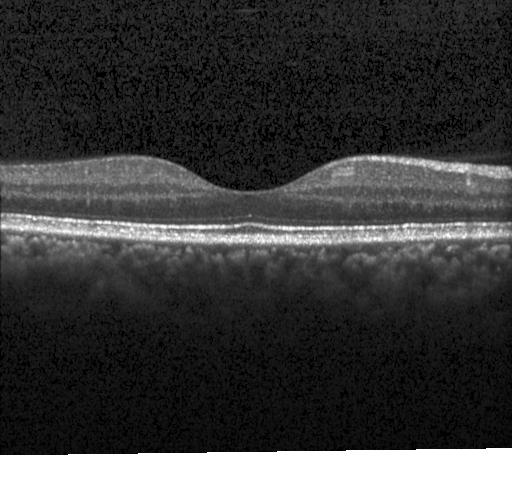 Heidelberg Spectralis OCT system. Optical coherence tomography scan — Assessment: neither choroidal neovascularization, diabetic macular edema, nor drusen.